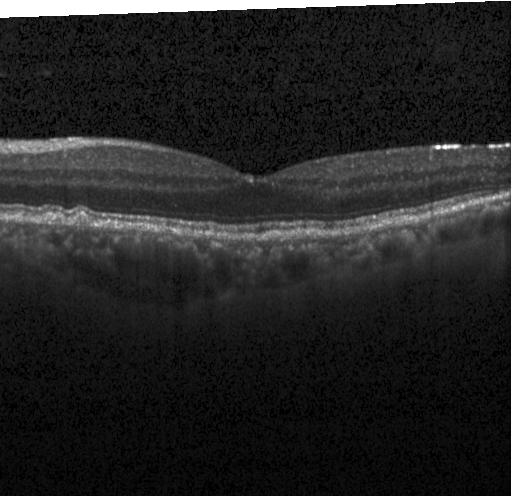 Horizontal scan through the fovea, spectral-domain optical coherence tomography, instrument: Heidelberg Spectralis, optical coherence tomography scan
Assessment: drusen.